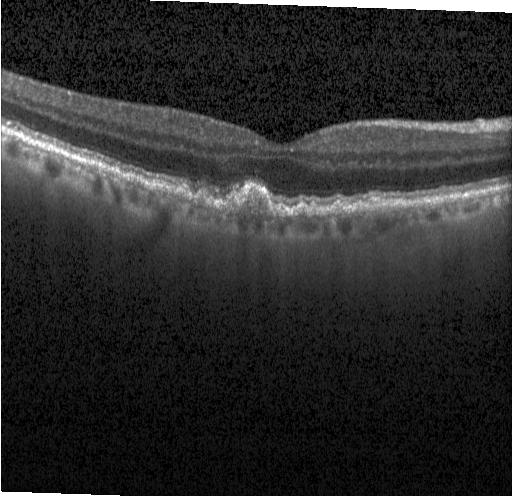
Through the macula · optical coherence tomography scan · Heidelberg Spectralis.
Dx: multiple drusen.